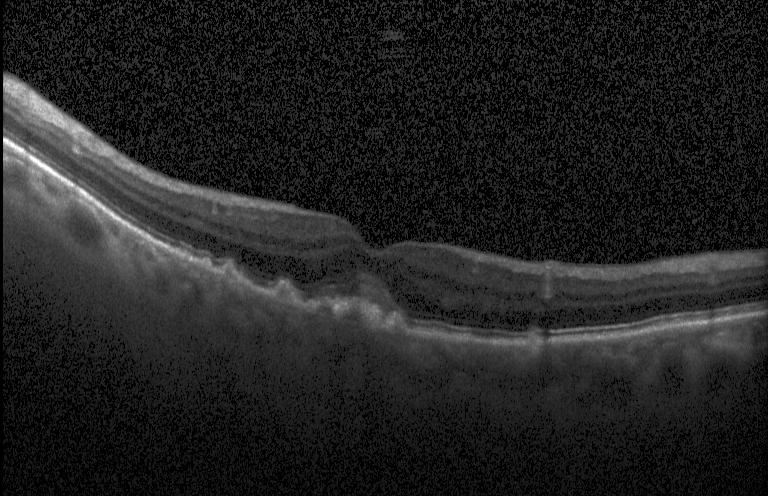
Assessment: choroidal neovascularization.